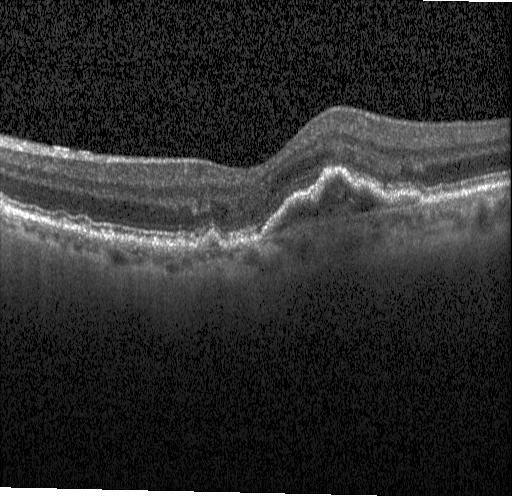

Retinal OCT cross-section, spectral-domain optical coherence tomography, fovea-centered, Heidelberg Spectralis. Impression: a choroidal neovascular membrane.